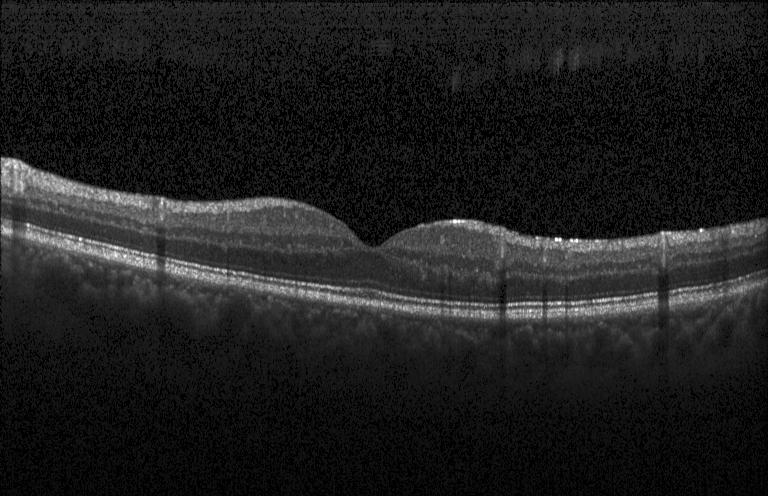

OCT finding: neither CNV, DME, nor drusen.